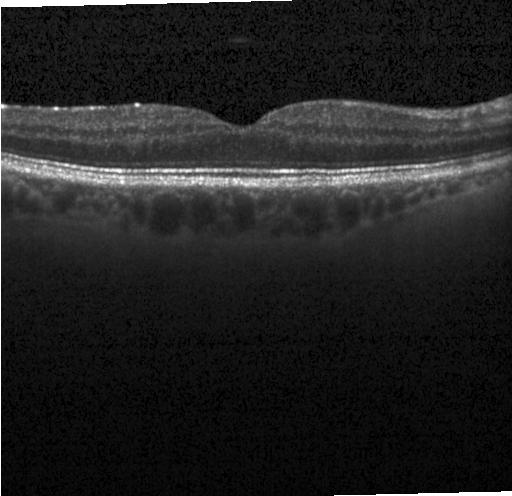
Impression: no evidence of CNV, DME, or drusen.